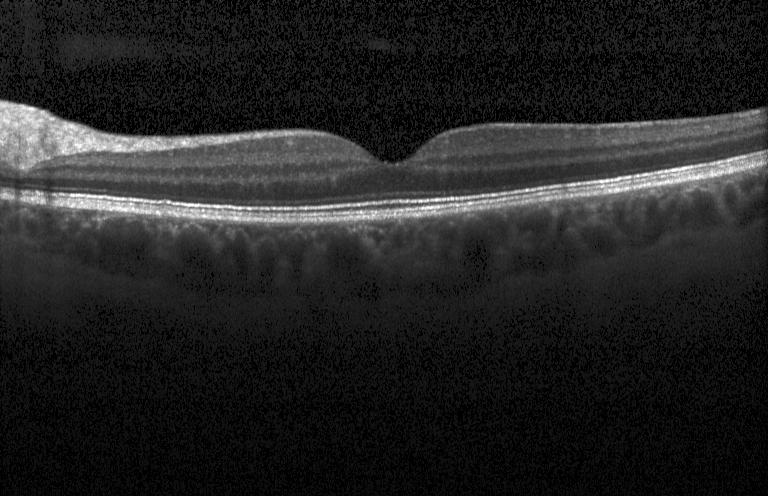
Spectral-domain OCT · macular scan · retinal OCT cross-section — No evidence of choroidal neovascularization, diabetic macular edema, or drusen.